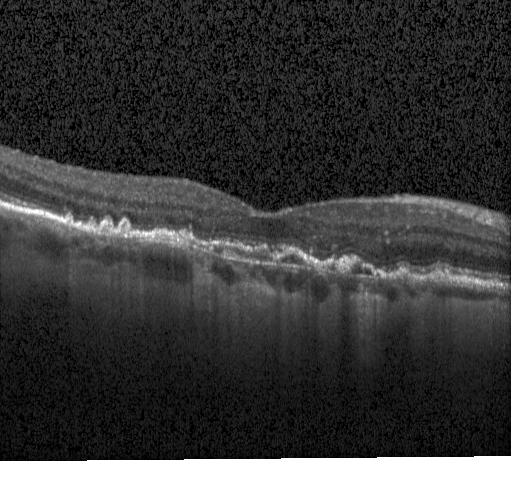 Horizontal scan through the fovea. Retinal OCT cross-section. Spectral-domain OCT. Impression: a choroidal neovascular membrane.